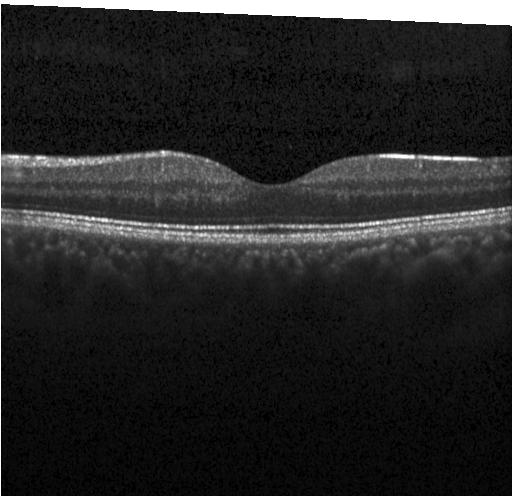
Acquired on a Heidelberg Spectralis · macular scan · optical coherence tomography scan. Macular OCT: no choroidal neovascularization, no diabetic macular edema, and no drusen.